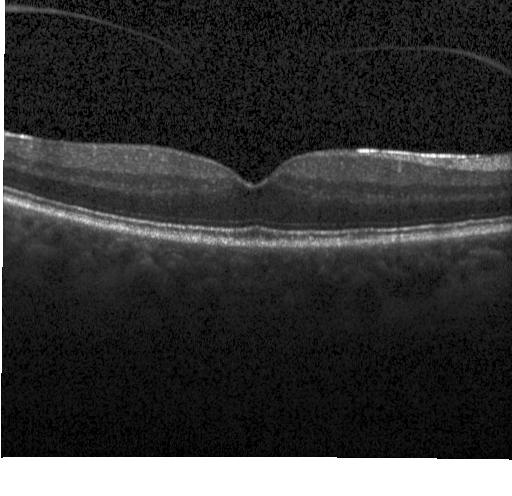
Retinal OCT cross-section.
Impression: no choroidal neovascularization, no diabetic macular edema, and no drusen.